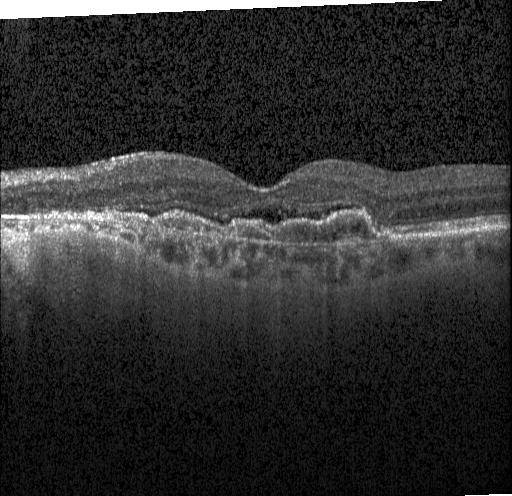
Macular OCT demonstrating a choroidal neovascular membrane.